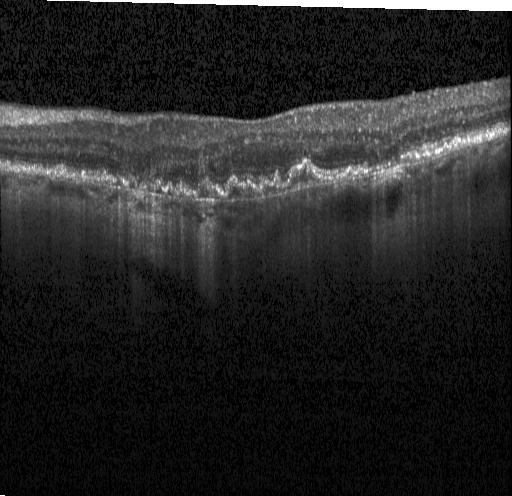 Macular OCT: choroidal neovascularization (CNV).